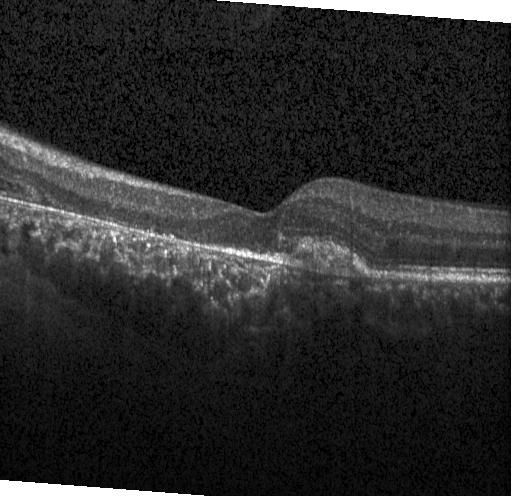 OCT line scan; through the macula; spectral-domain OCT — The scan shows a choroidal neovascular membrane.